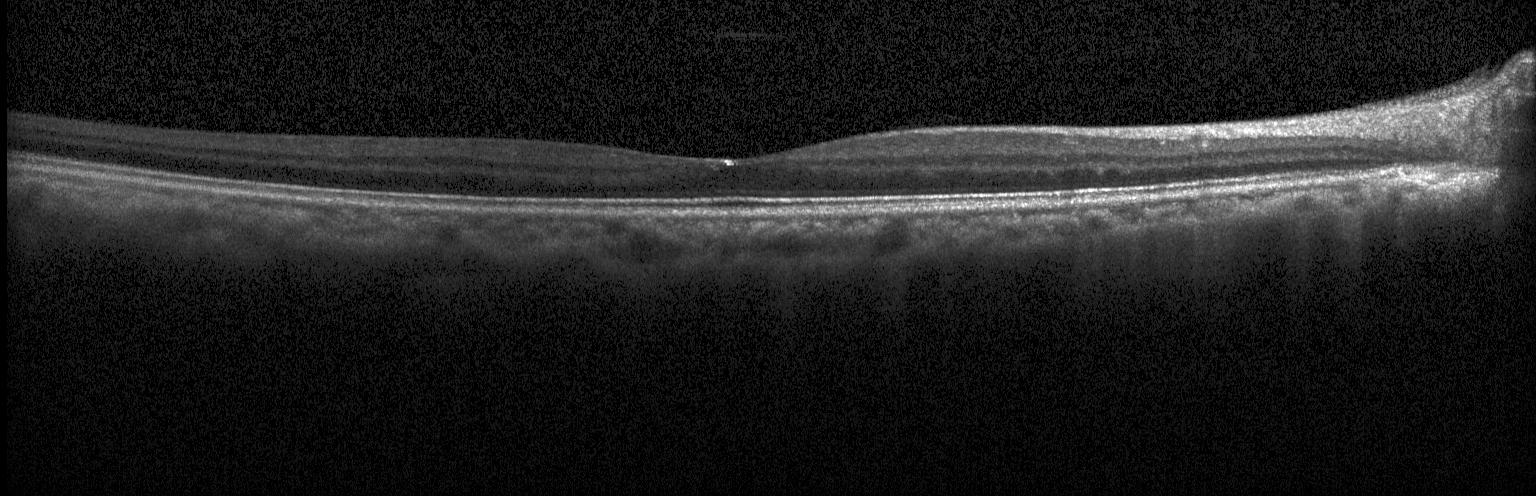
Horizontal scan through the fovea; optical coherence tomography scan; Heidelberg Spectralis; spectral-domain optical coherence tomography — Finding: no CNV, DME, or drusen.